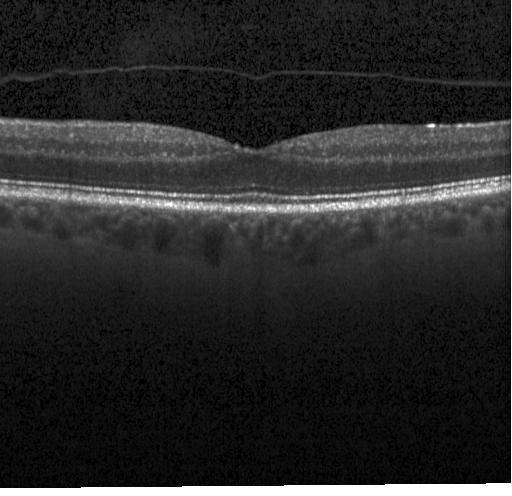

Spectral-domain OCT B-scan: no CNV, DME, or drusen.